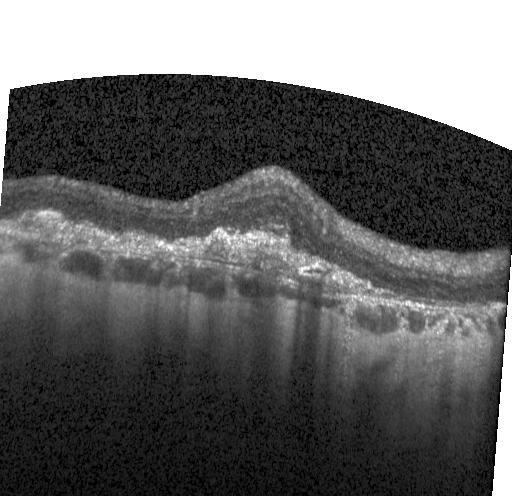 Heidelberg Spectralis OCT system, optical coherence tomography B-scan
This B-scan demonstrates CNV.